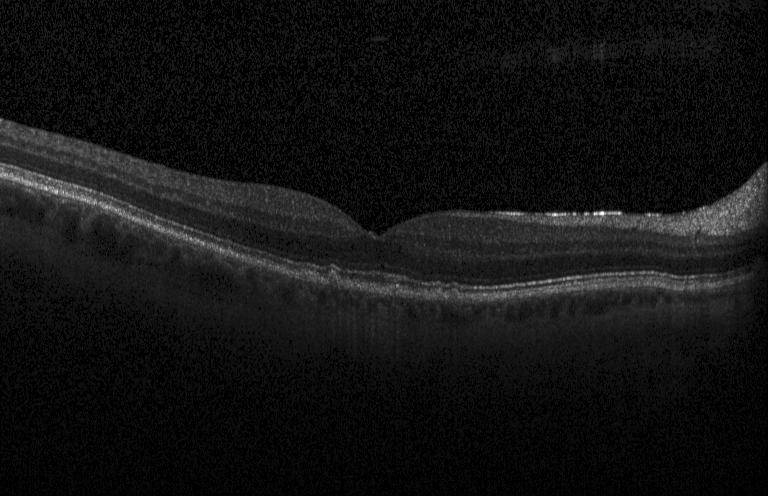 Impression: multiple drusen.